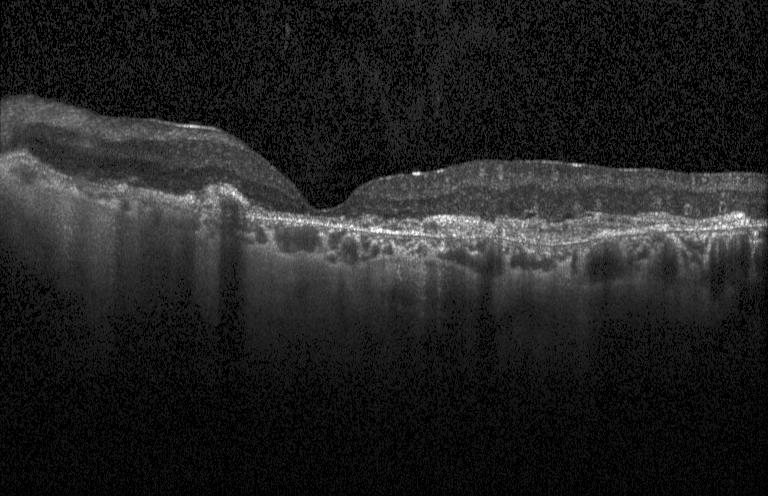

Retinal OCT cross-section
Finding: a choroidal neovascular membrane.